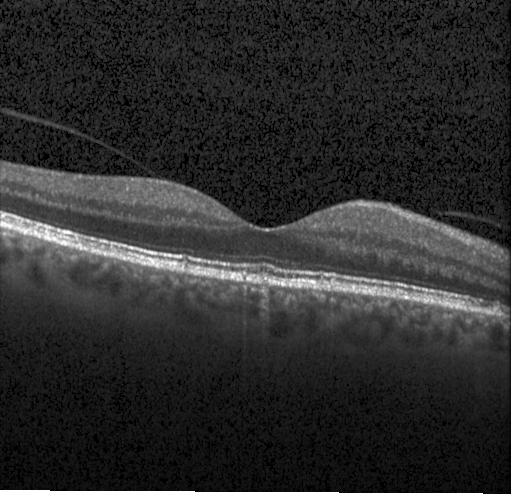

OCT finding: drusen.